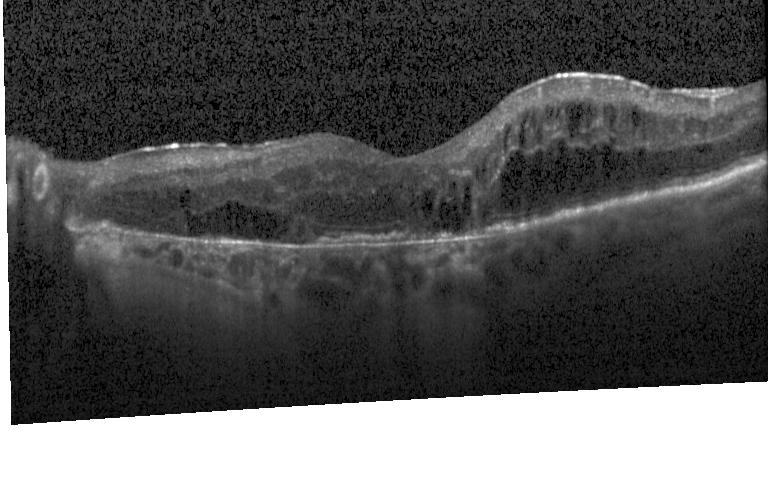

Macular scan. Retinal OCT B-scan. Acquired on a Heidelberg Spectralis. Spectral-domain optical coherence tomography — This B-scan demonstrates a choroidal neovascular membrane.